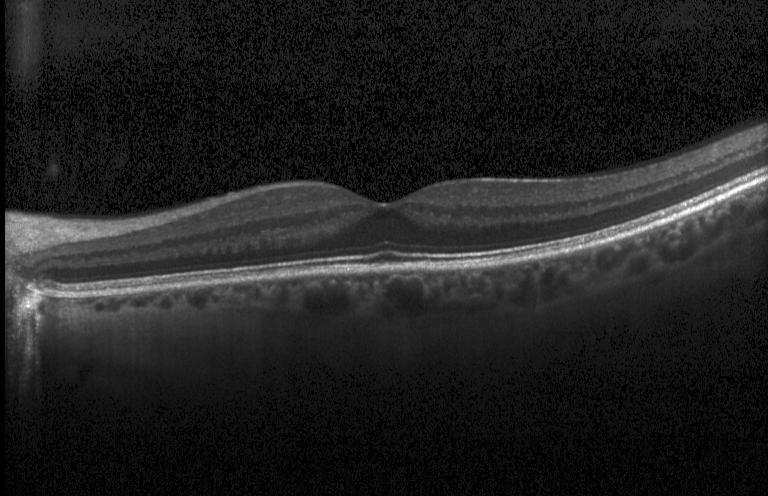

OCT B-scan.
Impression: no evidence of choroidal neovascularization, diabetic macular edema, or drusen.